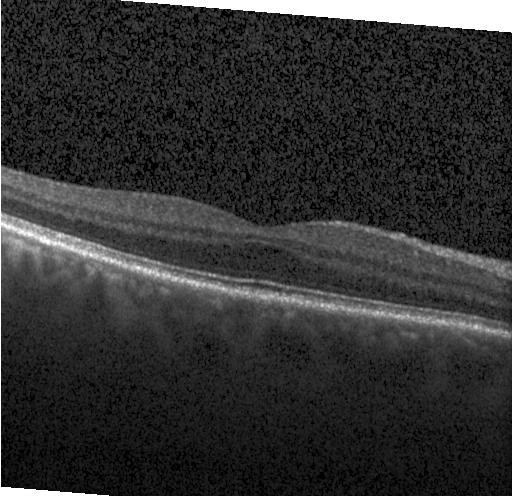 Retinal OCT B-scan. No choroidal neovascularization, no diabetic macular edema, and no drusen.